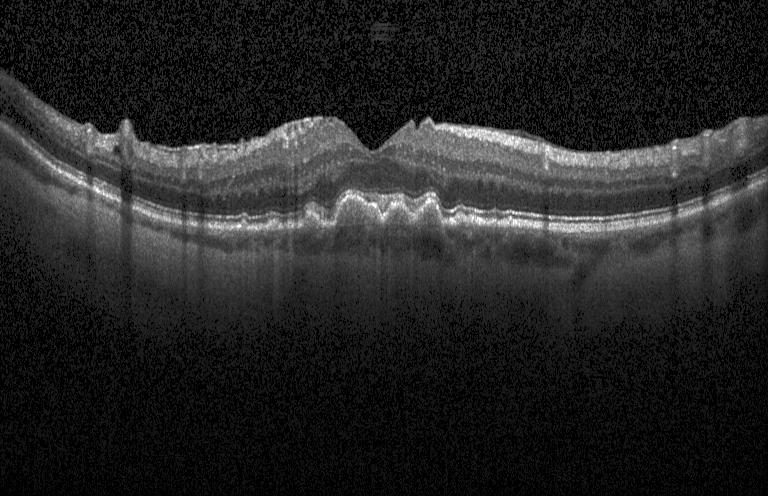 SD-OCT · instrument: Heidelberg Spectralis · retinal OCT B-scan · centered on the fovea
Diagnosis: multiple drusen.